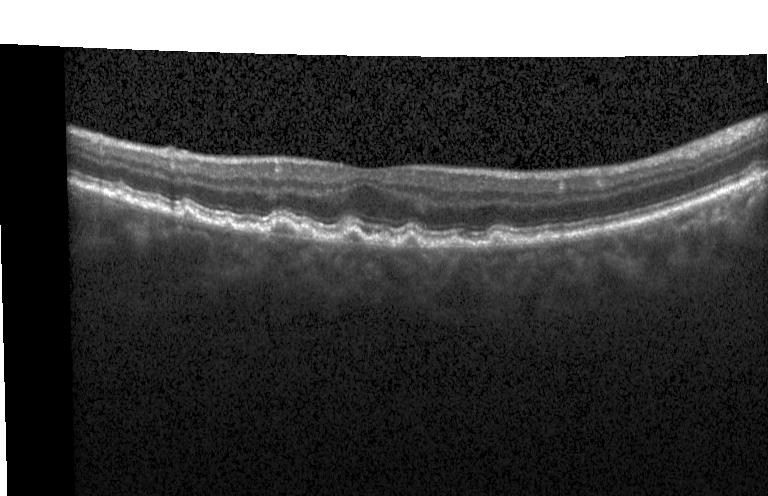

Heidelberg Spectralis OCT system; spectral-domain OCT; OCT line scan — Multiple drusen.